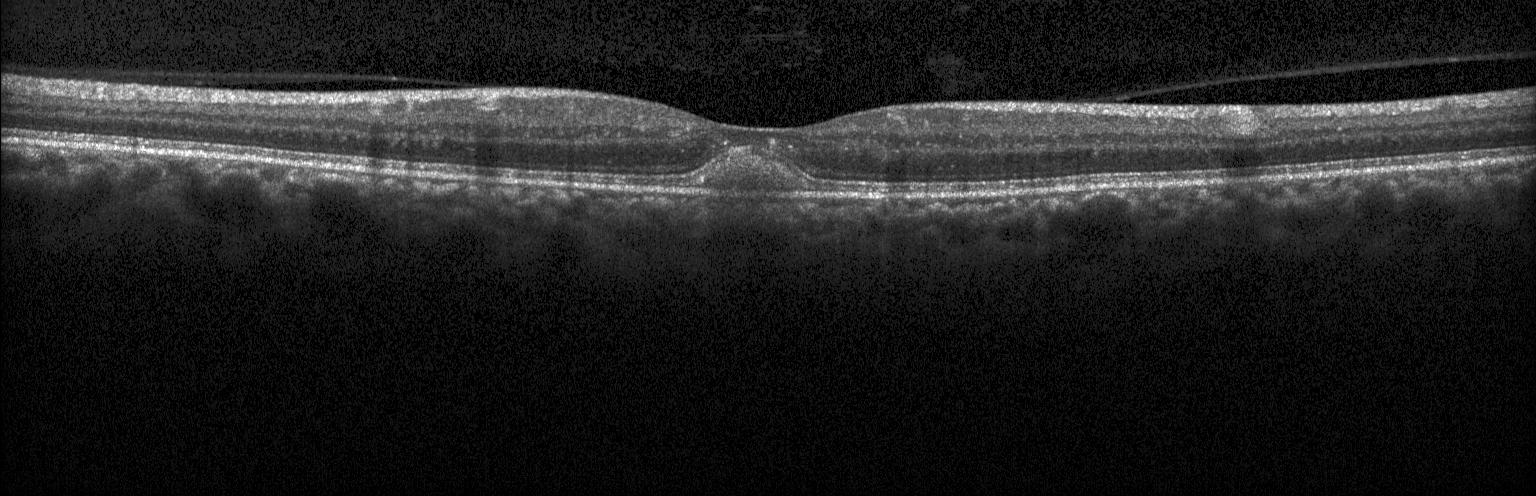

OCT B-scan showing a choroidal neovascular membrane.